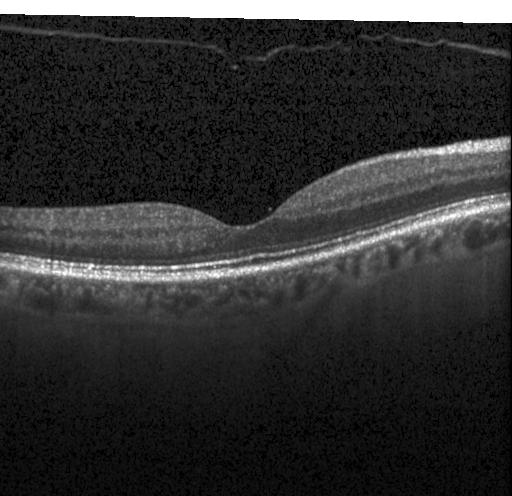 Retinal OCT B-scan.
Assessment: no CNV, DME, or drusen.